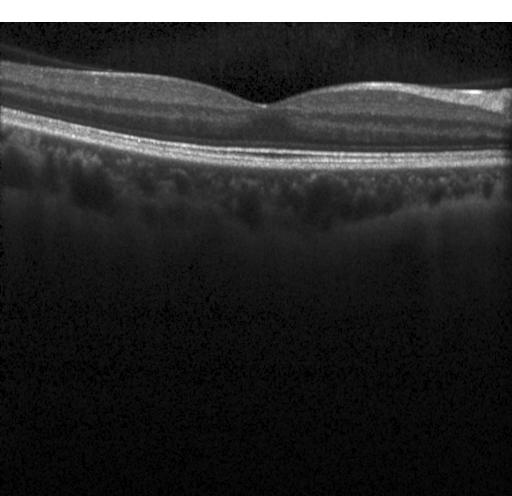 Optical coherence tomography B-scan. Impression: neither choroidal neovascularization, diabetic macular edema, nor drusen.